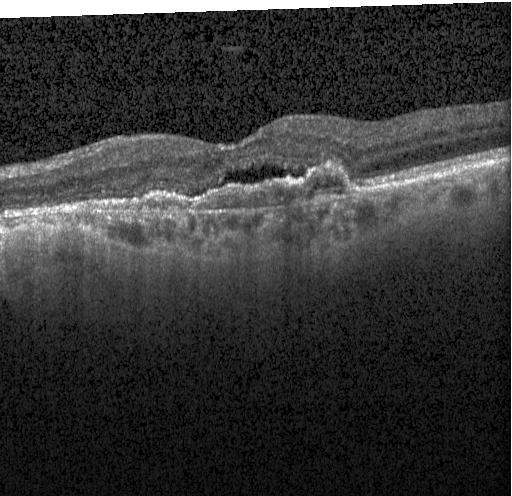

OCT B-scan showing choroidal neovascularization (CNV).